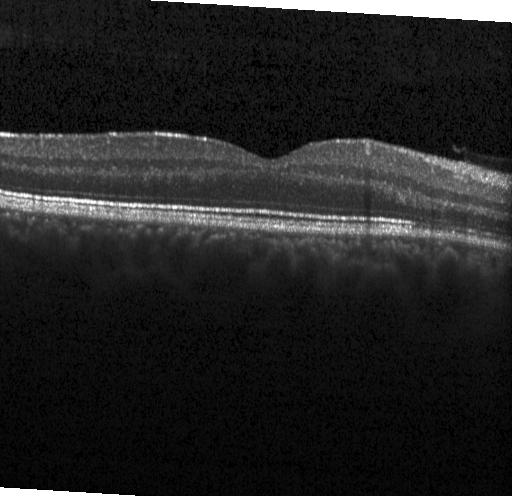
Dx: neither choroidal neovascularization, diabetic macular edema, nor drusen.